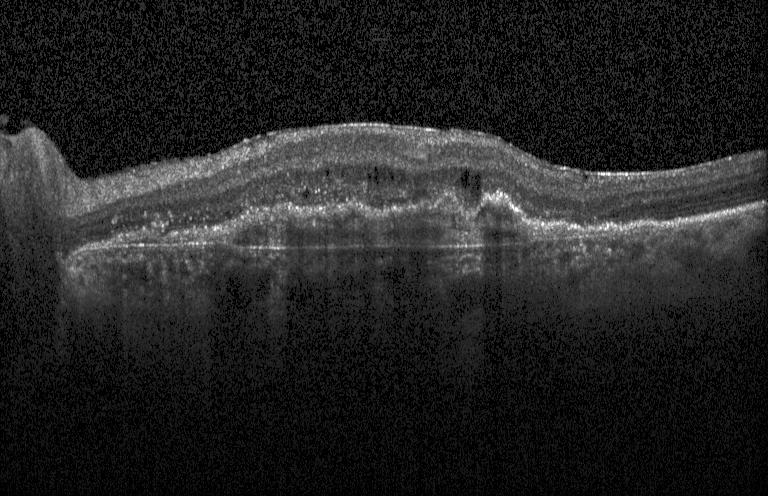
This B-scan demonstrates choroidal neovascularization (CNV).